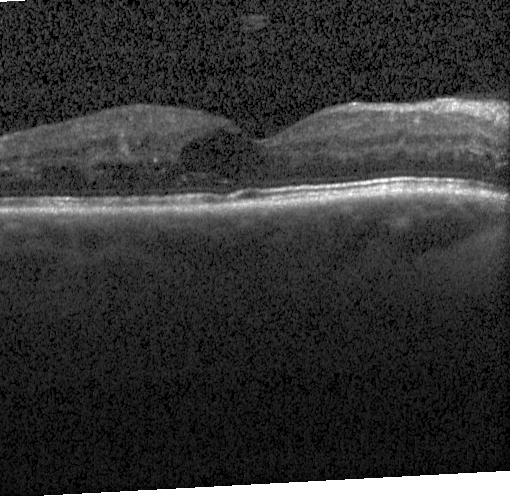
OCT line scan, instrument: Heidelberg Spectralis — Diabetic macular edema (DME).